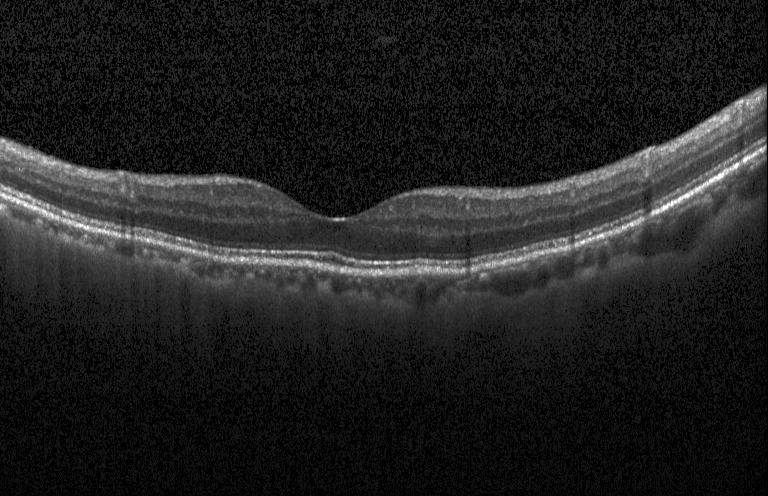
Finding: no CNV, DME, or drusen.